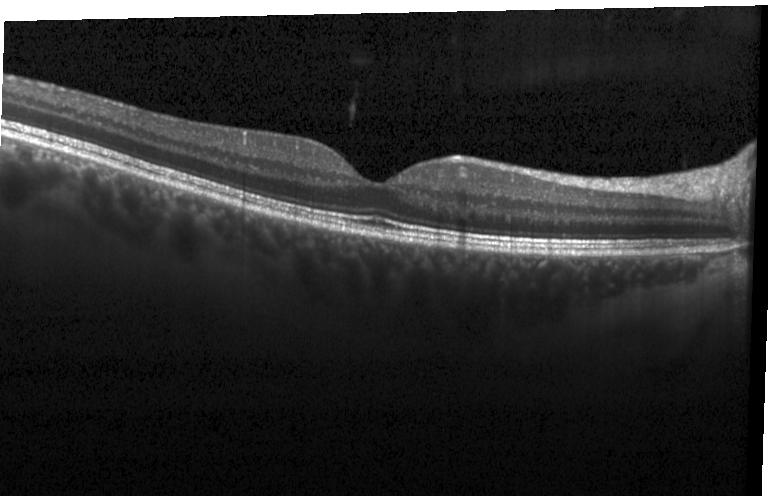
Retinal OCT cross-section — Macular OCT: no choroidal neovascularization, diabetic macular edema, or drusen.